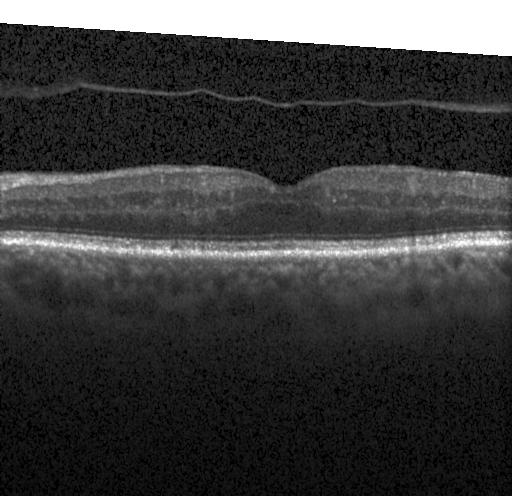

Retinal OCT B-scan.
Diagnosis: no CNV, DME, or drusen.